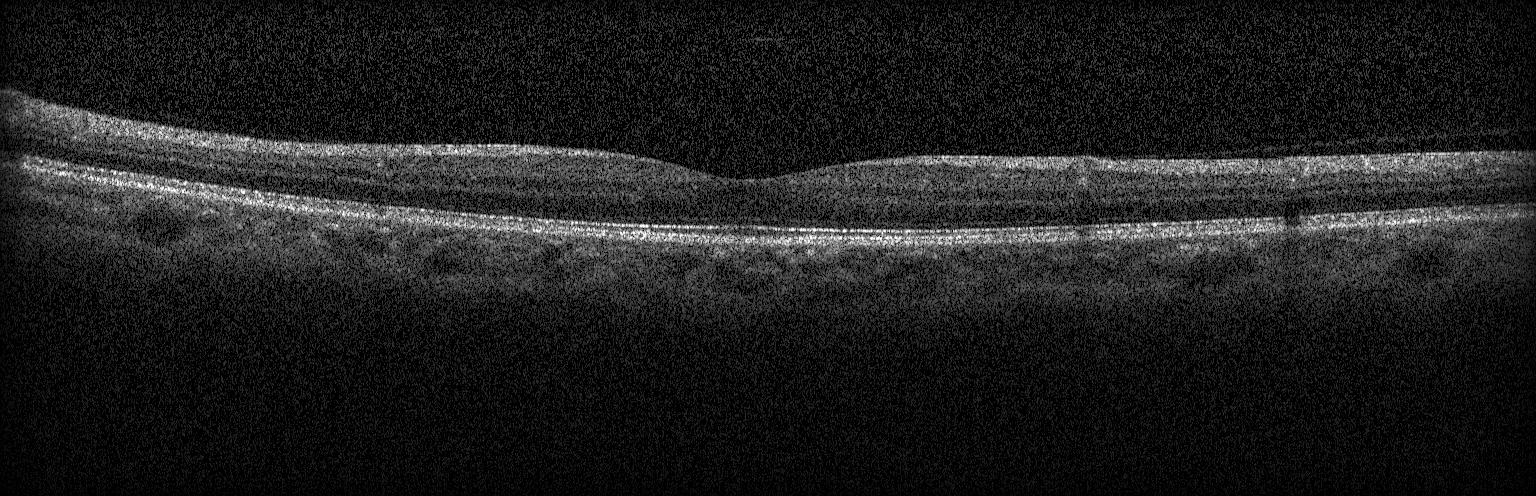

Horizontal scan through the fovea, OCT B-scan — Dx: no CNV, no DME, and no drusen.